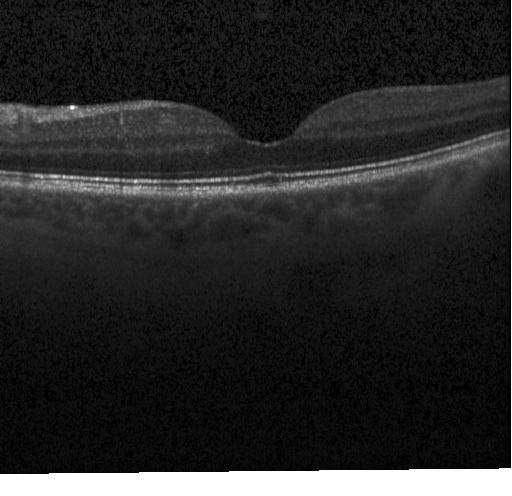 Dx: no evidence of CNV, DME, or drusen.